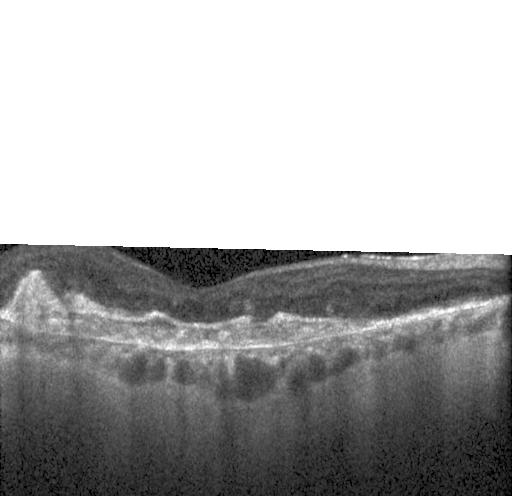 Assessment: choroidal neovascularization (CNV).